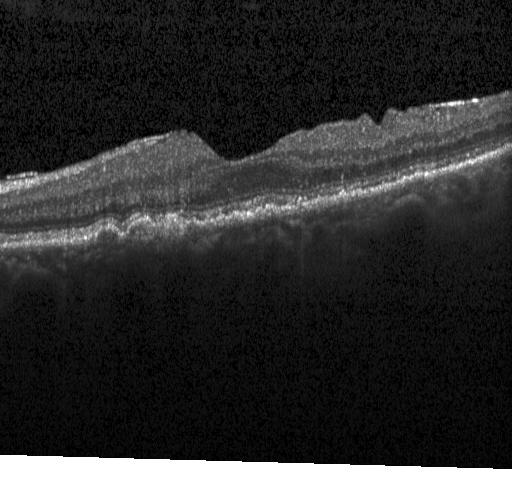

Instrument: Heidelberg Spectralis, spectral-domain optical coherence tomography, macular scan, OCT B-scan
Impression: multiple drusen.